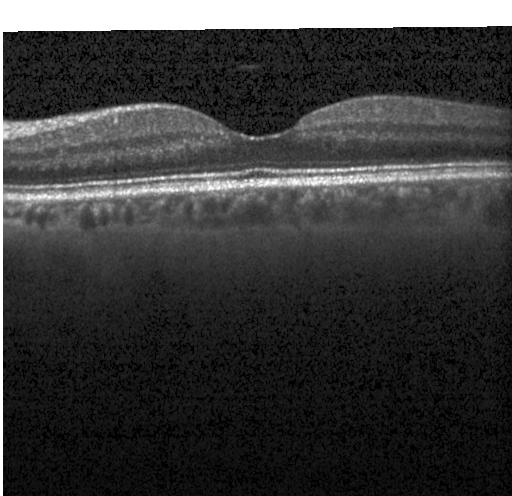

OCT line scan · instrument: Heidelberg Spectralis
Finding: neither choroidal neovascularization, diabetic macular edema, nor drusen.